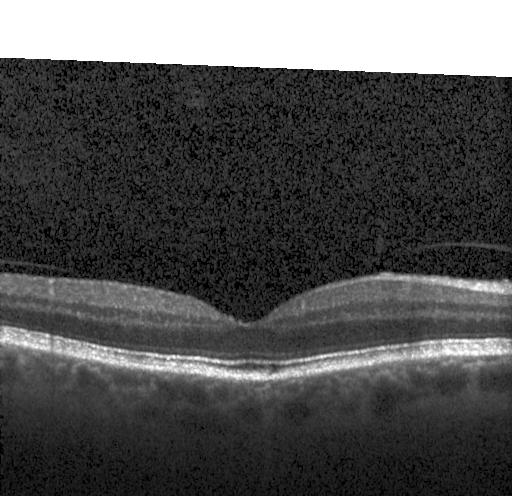

Heidelberg Spectralis, optical coherence tomography scan, fovea-centered, spectral-domain OCT — Impression: neither choroidal neovascularization, diabetic macular edema, nor drusen.